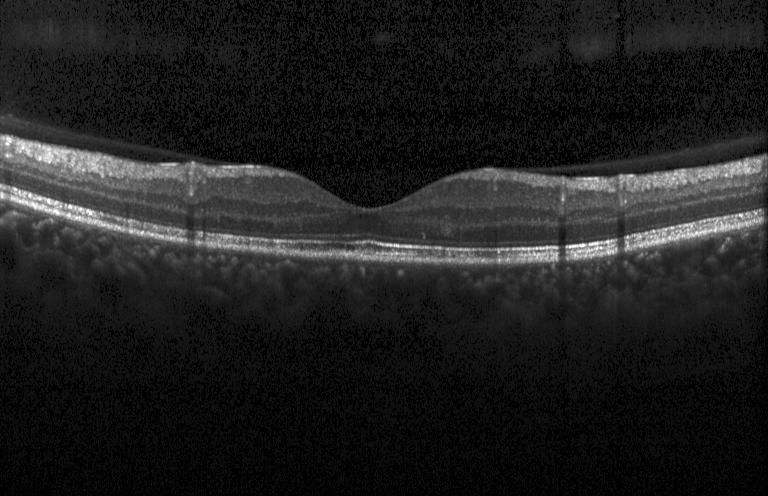 Retinal OCT B-scan; spectral-domain optical coherence tomography; horizontal scan through the fovea; Heidelberg Spectralis OCT system
OCT finding: no choroidal neovascularization, no diabetic macular edema, and no drusen.